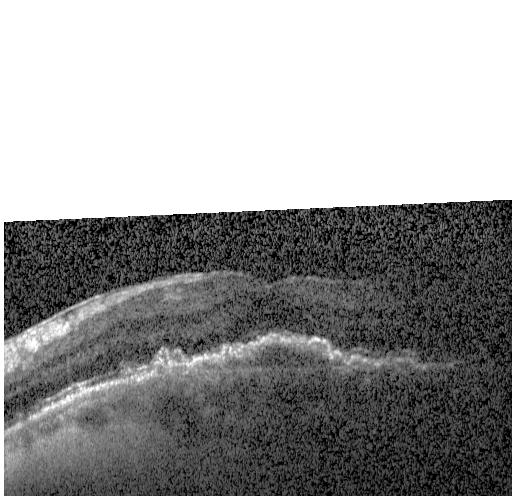
Optical coherence tomography scan — Diagnosis: choroidal neovascularization (CNV).